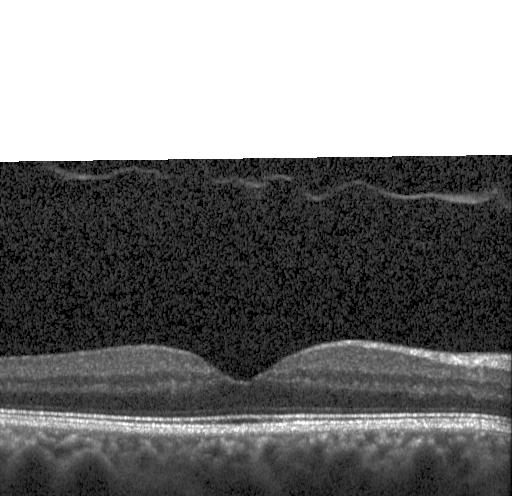 Spectral-domain OCT B-scan: no choroidal neovascularization, no diabetic macular edema, and no drusen.